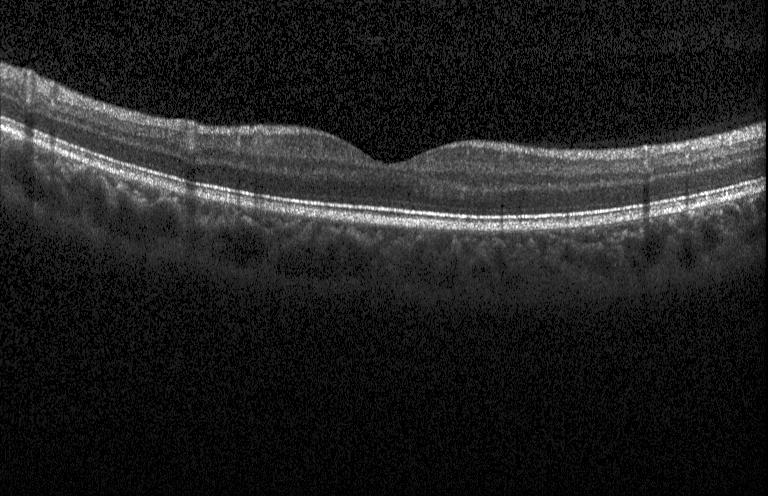
Dx: neither choroidal neovascularization, diabetic macular edema, nor drusen.